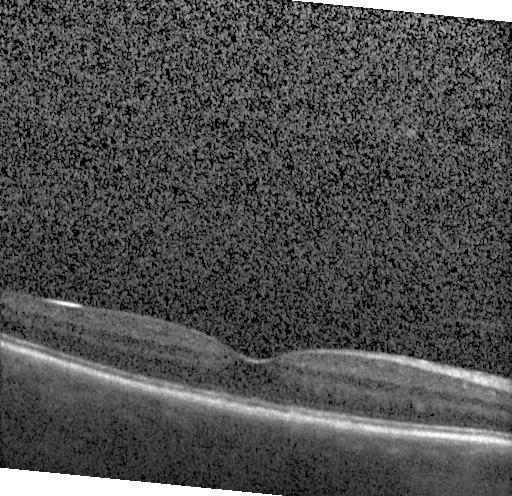
OCT line scan; SD-OCT.
Finding: neither choroidal neovascularization, diabetic macular edema, nor drusen.